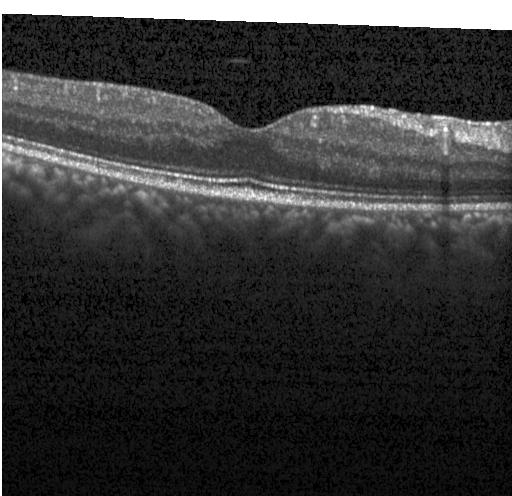

OCT finding: no evidence of choroidal neovascularization, diabetic macular edema, or drusen.